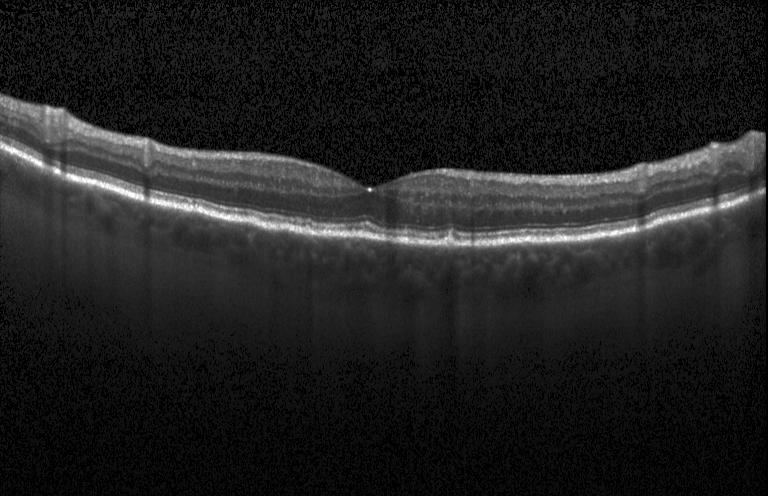
Diagnosis: multiple drusen.